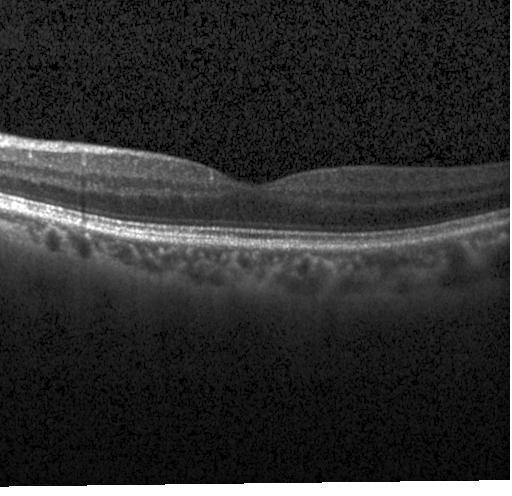 Fovea-centered · OCT B-scan · SD-OCT. Finding: no evidence of choroidal neovascularization, diabetic macular edema, or drusen.